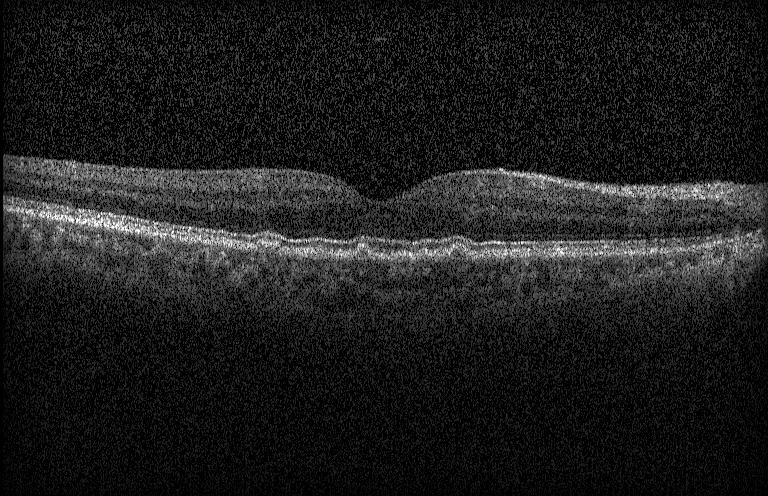 Heidelberg Spectralis, optical coherence tomography B-scan
Diagnosis: multiple drusen.